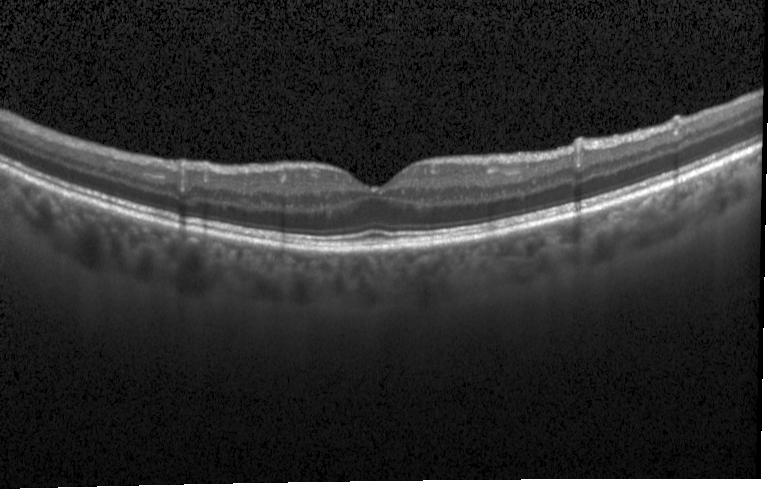 Dx: no choroidal neovascularization, diabetic macular edema, or drusen.